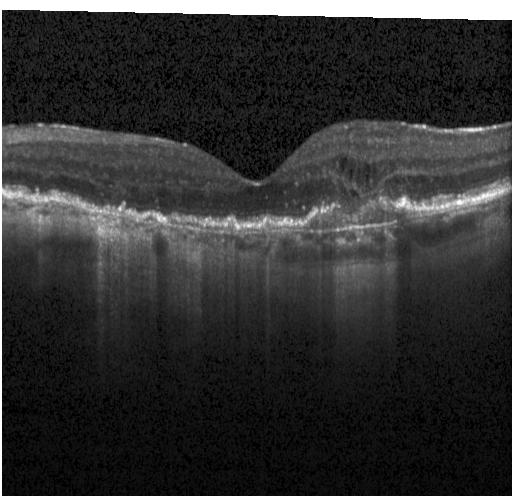

Macular OCT: a choroidal neovascular membrane.